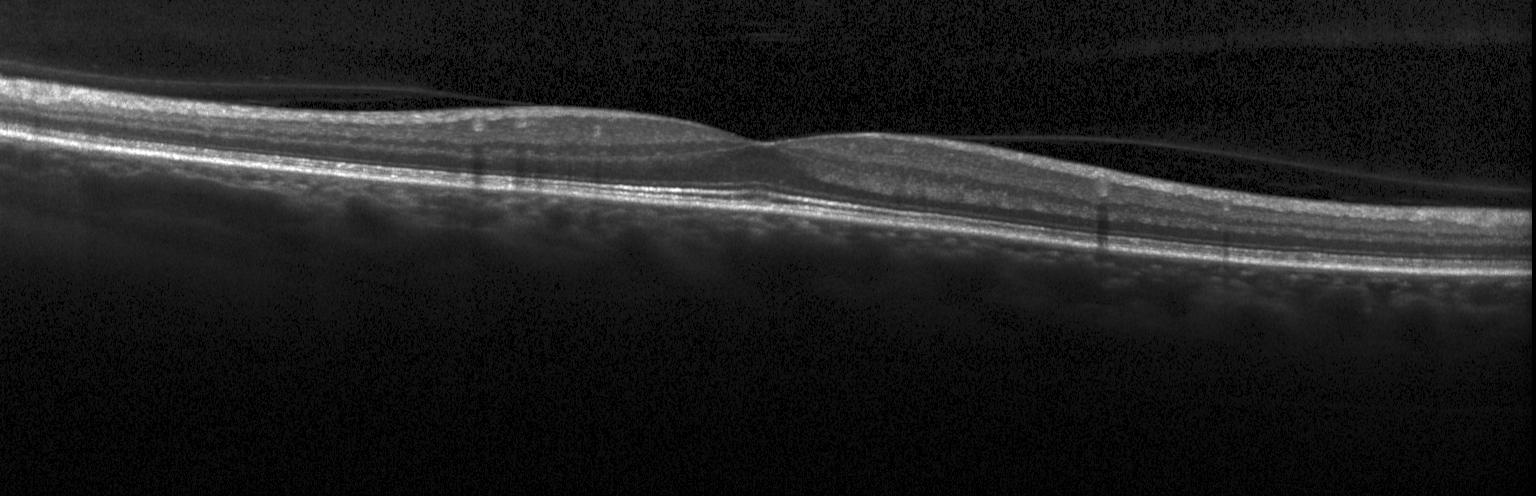

Heidelberg Spectralis OCT system · retinal OCT B-scan · macular scan. Assessment: no choroidal neovascularization, diabetic macular edema, or drusen.